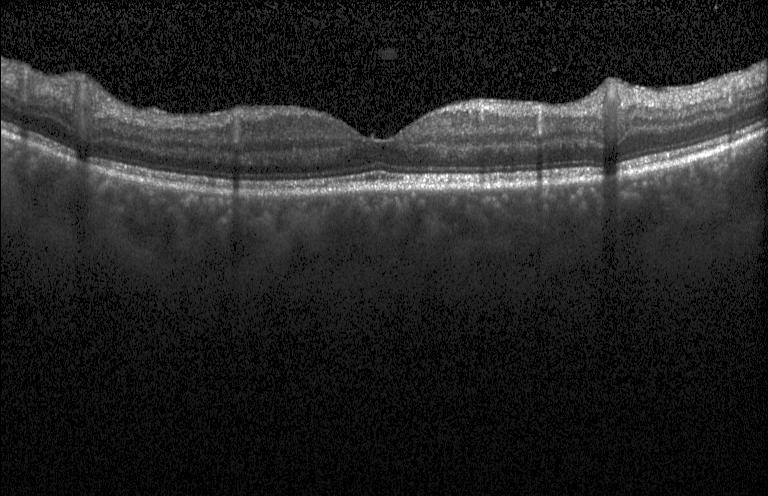
Spectral-domain OCT B-scan: neither choroidal neovascularization, diabetic macular edema, nor drusen.